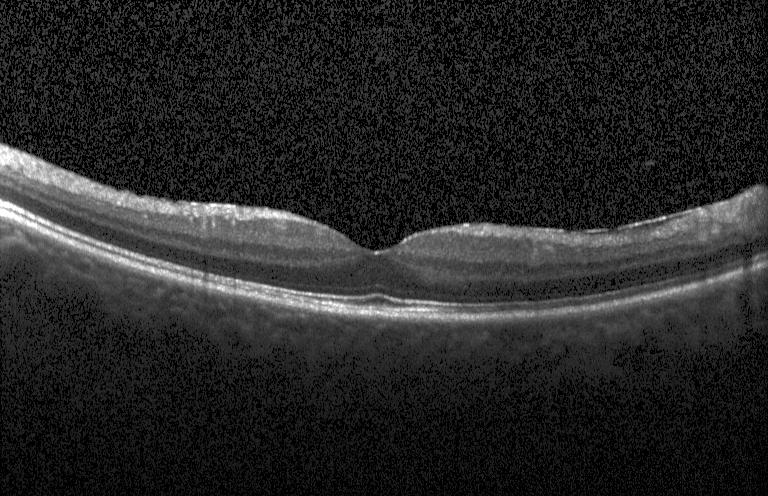 OCT B-scan — Impression: no evidence of choroidal neovascularization, diabetic macular edema, or drusen.